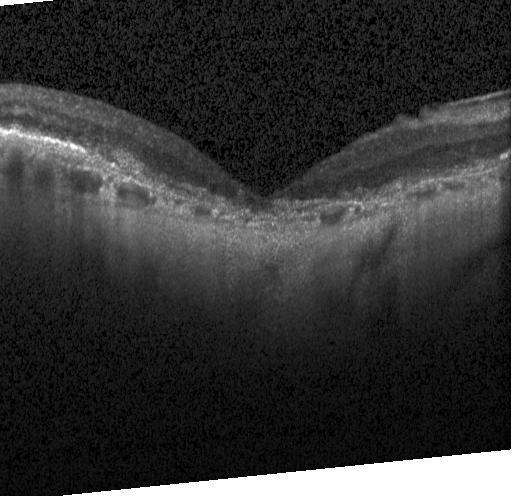 Instrument: Heidelberg Spectralis · retinal OCT B-scan.
This B-scan demonstrates CNV.